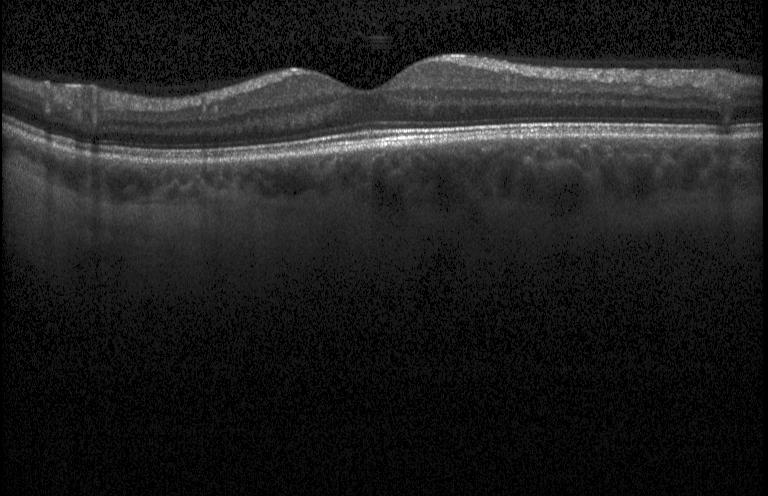

Spectral-domain optical coherence tomography; macular scan; optical coherence tomography scan. Diagnosis: no choroidal neovascularization, no diabetic macular edema, and no drusen.